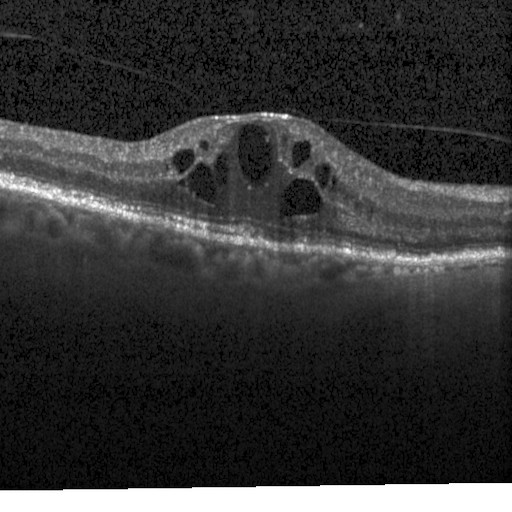
Heidelberg Spectralis. Optical coherence tomography B-scan. Through the macula. SD-OCT.
This B-scan demonstrates diabetic macular edema.